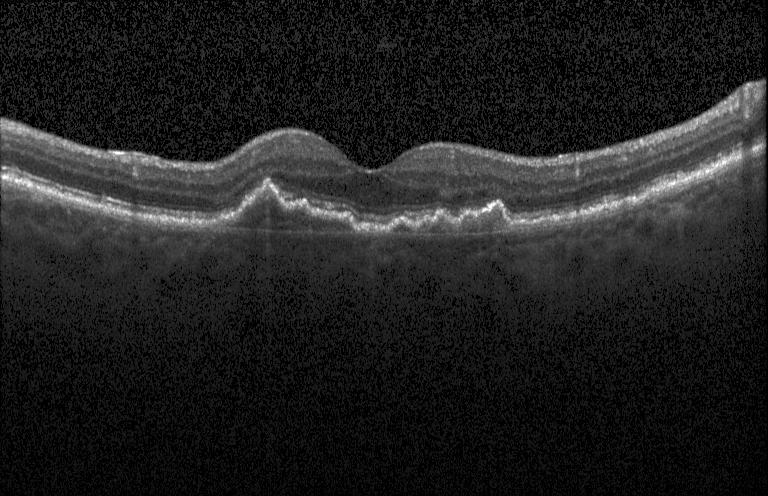

OCT finding: a choroidal neovascular membrane.